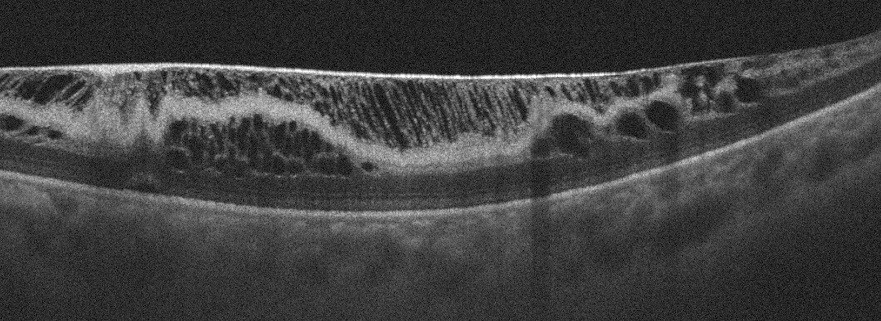
ERM.